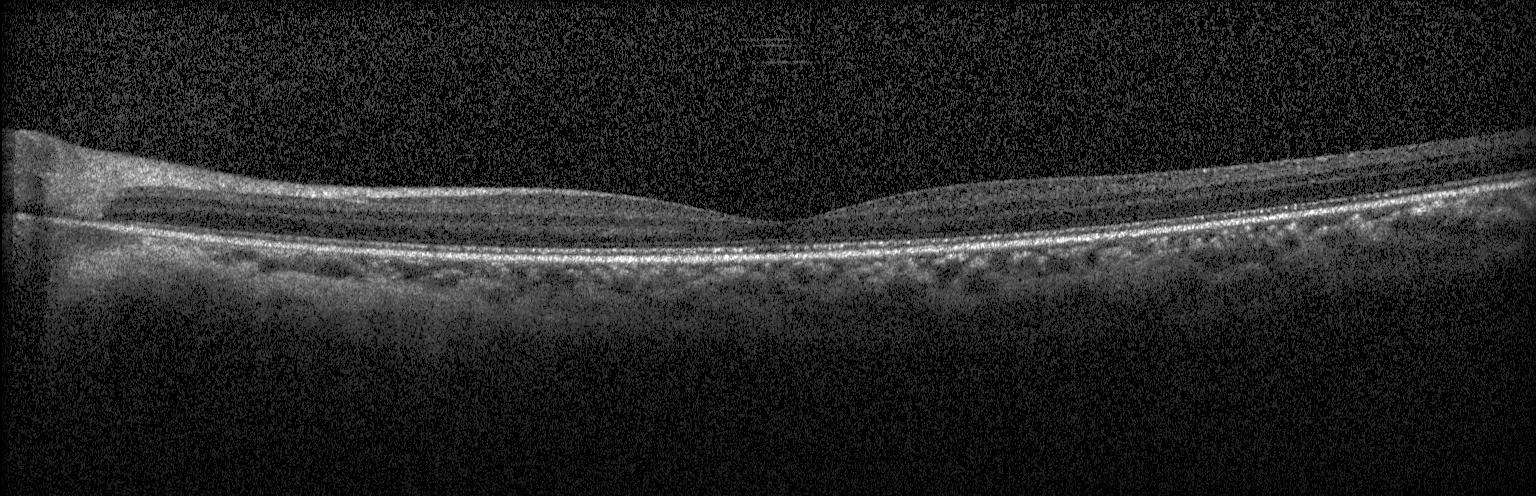 Retinal OCT cross-section, instrument: Heidelberg Spectralis, spectral-domain optical coherence tomography.
Impression: neither choroidal neovascularization, diabetic macular edema, nor drusen.